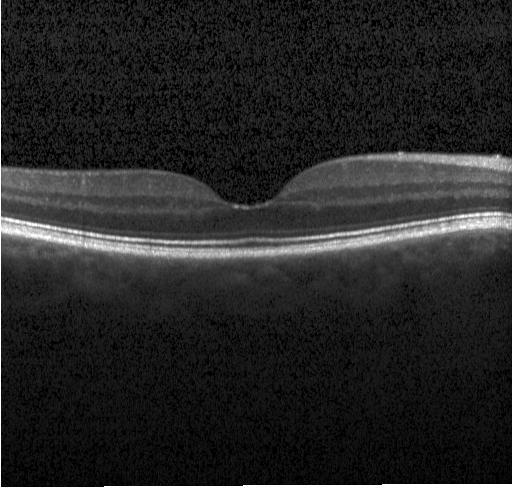
OCT finding: no CNV, no DME, and no drusen.